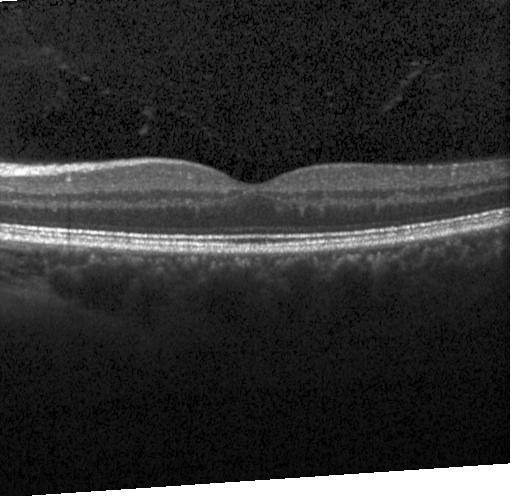

Impression: no evidence of CNV, DME, or drusen.